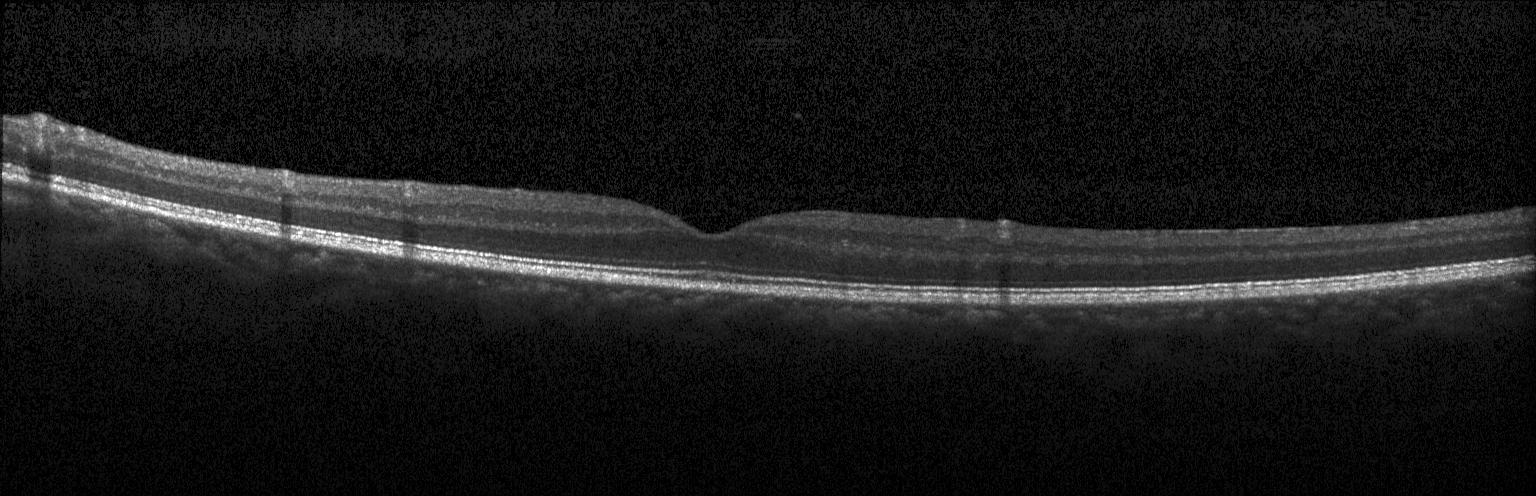 OCT B-scan. Centered on the fovea. Heidelberg Spectralis OCT system. OCT finding: no CNV, no DME, and no drusen.